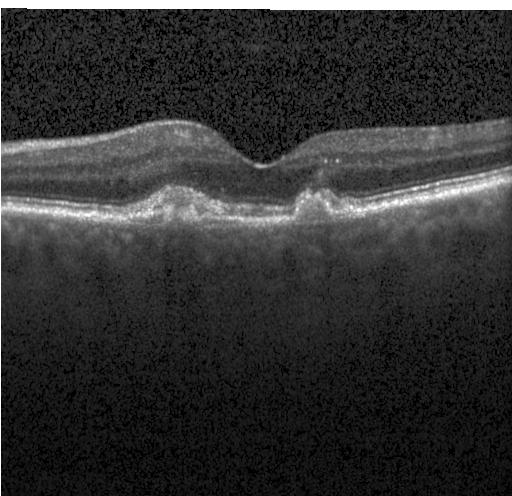 Optical coherence tomography B-scan. Assessment: CNV.